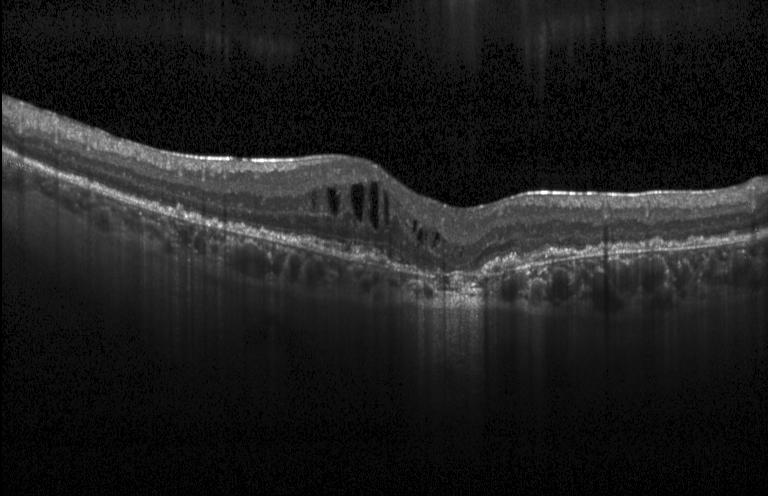
Retinal OCT B-scan, spectral-domain optical coherence tomography, acquired on a Heidelberg Spectralis
Assessment: a choroidal neovascular membrane.